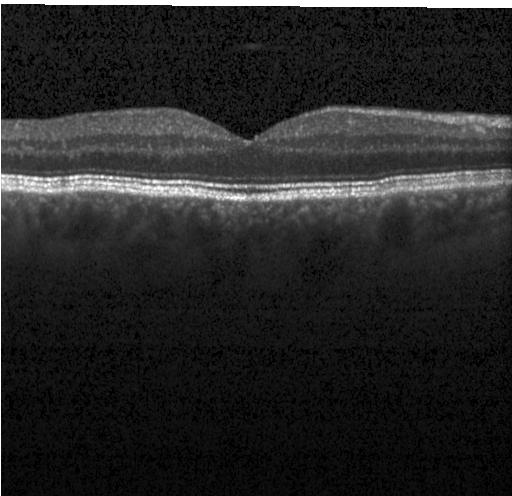
OCT B-scan · spectral-domain optical coherence tomography · acquired on a Heidelberg Spectralis. This B-scan demonstrates neither choroidal neovascularization, diabetic macular edema, nor drusen.